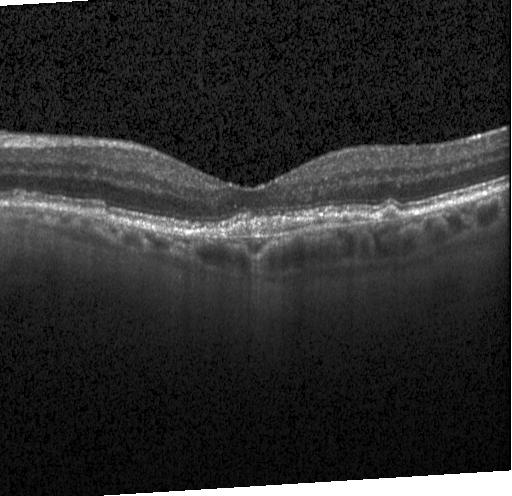 Heidelberg Spectralis OCT system · retinal OCT B-scan · SD-OCT. Diagnosis: a choroidal neovascular membrane.